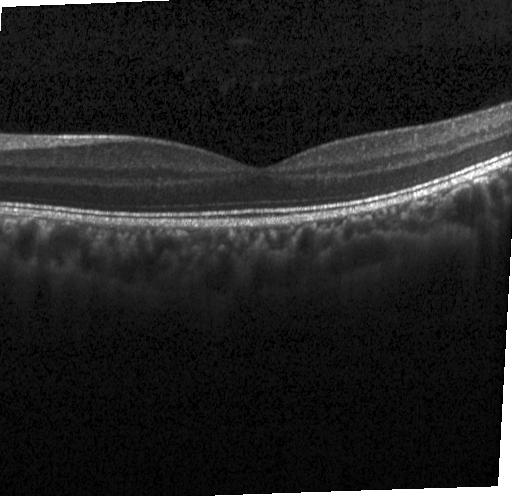

OCT line scan, spectral-domain OCT, Heidelberg Spectralis.
Macular OCT: neither choroidal neovascularization, diabetic macular edema, nor drusen.